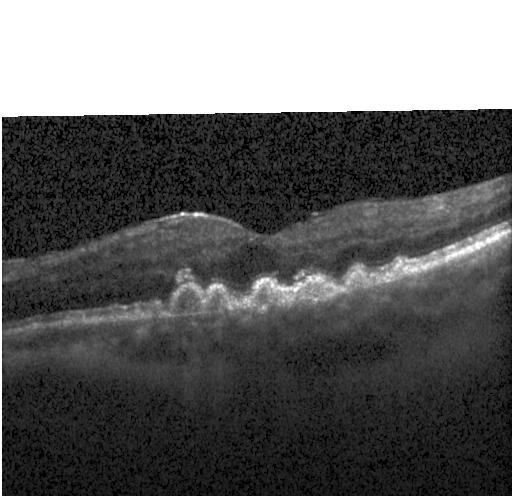

Spectral-domain OCT B-scan: multiple drusen.